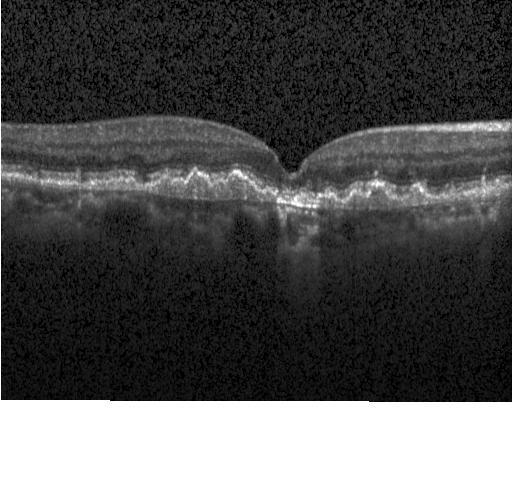

Heidelberg Spectralis · spectral-domain OCT · macular scan · retinal OCT cross-section. Diagnosis: choroidal neovascularization (CNV).